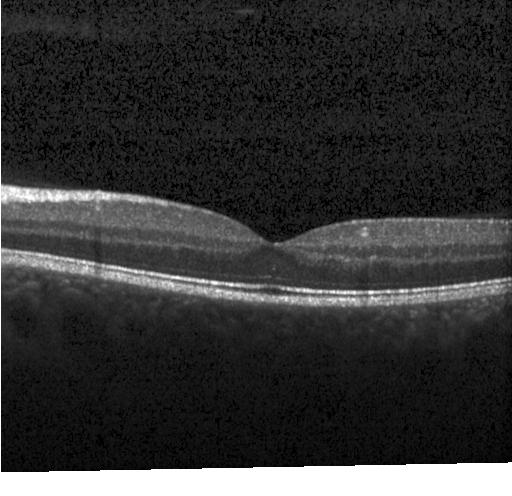
Horizontal scan through the fovea. Spectral-domain optical coherence tomography. Retinal OCT cross-section. Heidelberg Spectralis
The scan shows no evidence of choroidal neovascularization, diabetic macular edema, or drusen.